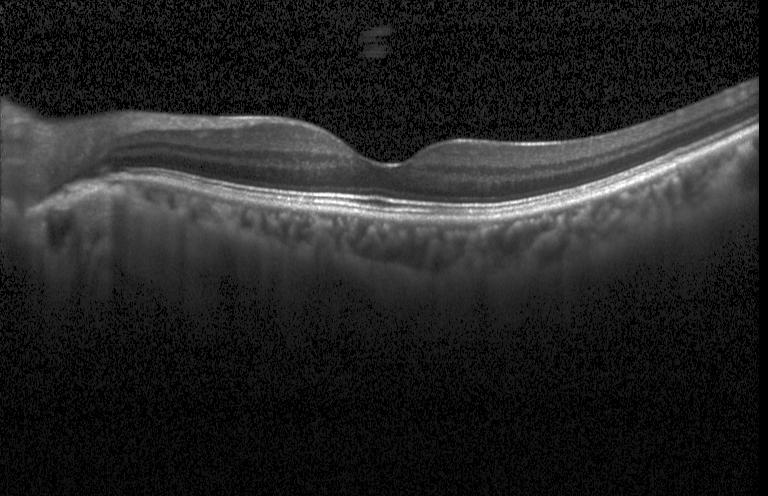 Fovea-centered, retinal OCT cross-section
The scan shows neither choroidal neovascularization, diabetic macular edema, nor drusen.